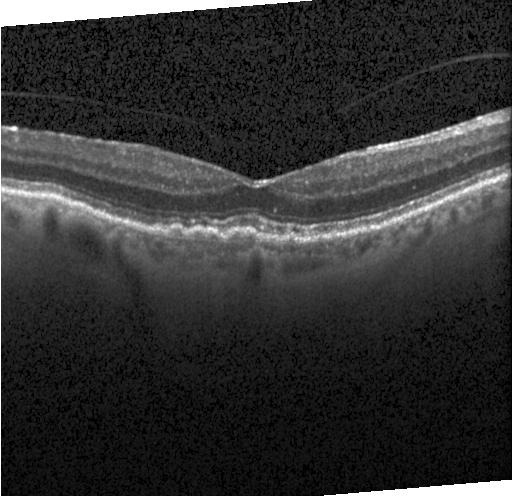

OCT line scan. Fovea-centered.
Finding: sub-RPE drusenoid deposits.